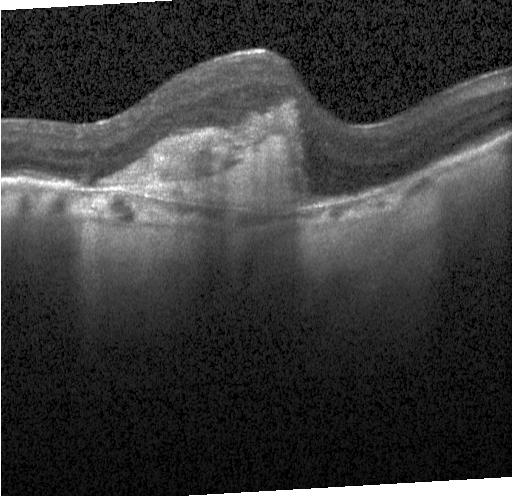

Dx: CNV.